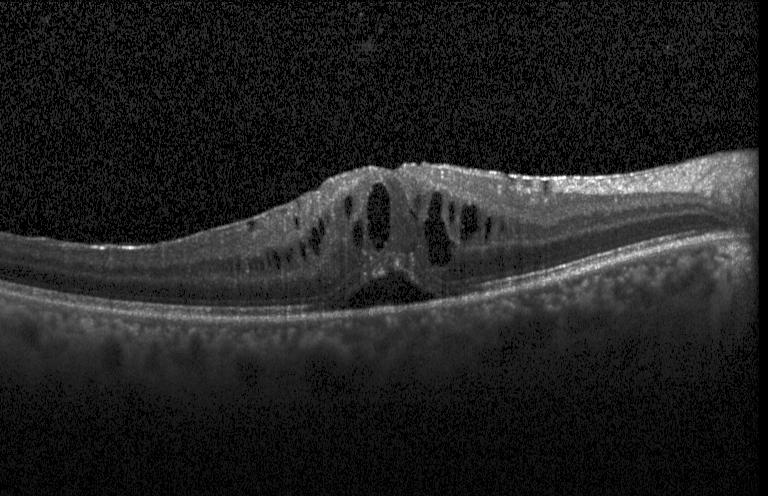 Retinal OCT cross-section.
Finding: DME.